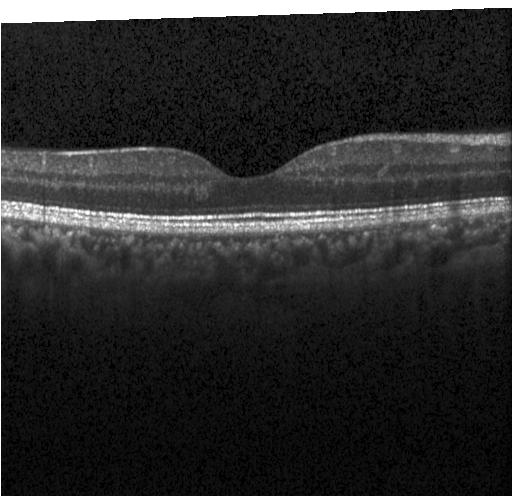
OCT finding: no CNV, no DME, and no drusen.